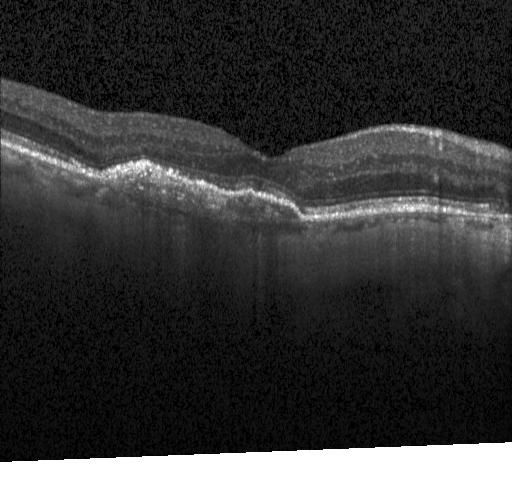

Heidelberg Spectralis OCT system; optical coherence tomography B-scan; horizontal scan through the fovea.
Finding: CNV.